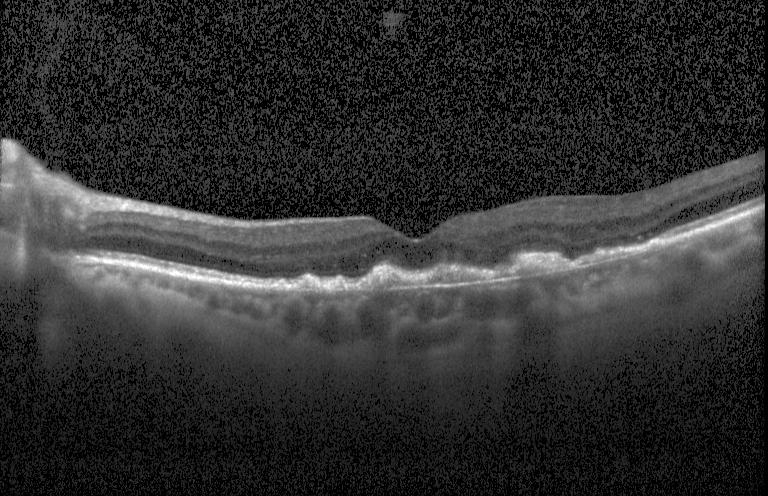 Horizontal scan through the fovea, Heidelberg Spectralis, retinal OCT B-scan
Impression: a choroidal neovascular membrane.